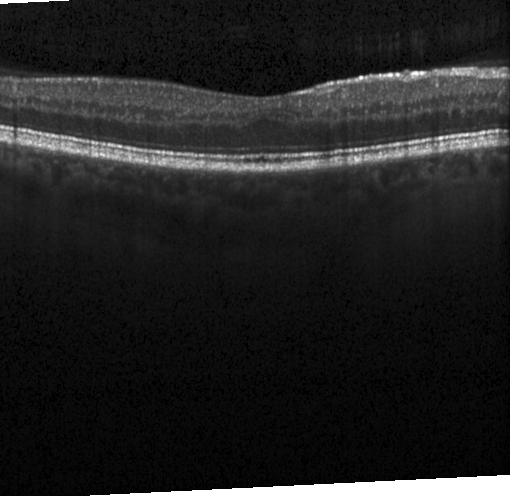 OCT scan showing neither choroidal neovascularization, diabetic macular edema, nor drusen.